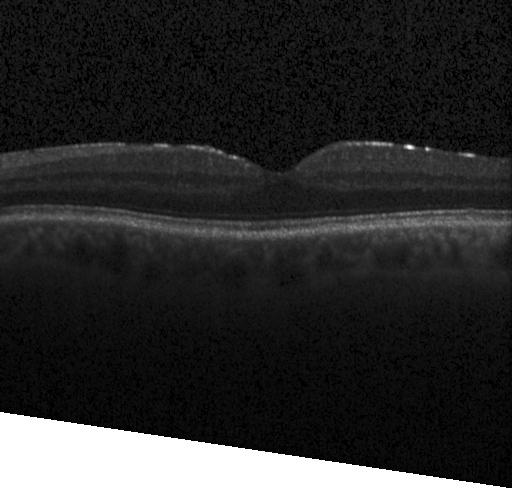

Optical coherence tomography scan. Heidelberg Spectralis OCT system.
Diagnosis: no CNV, DME, or drusen.